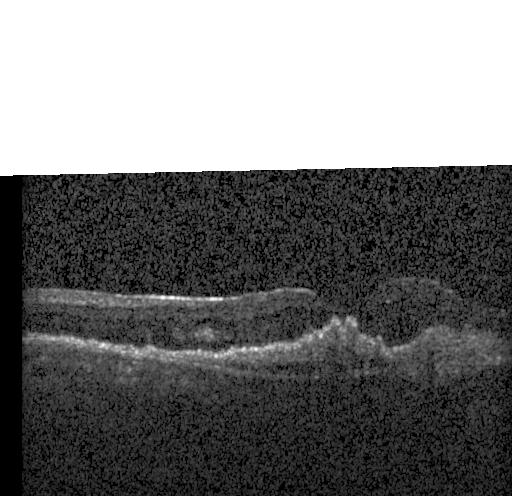
Diagnosis: a choroidal neovascular membrane.